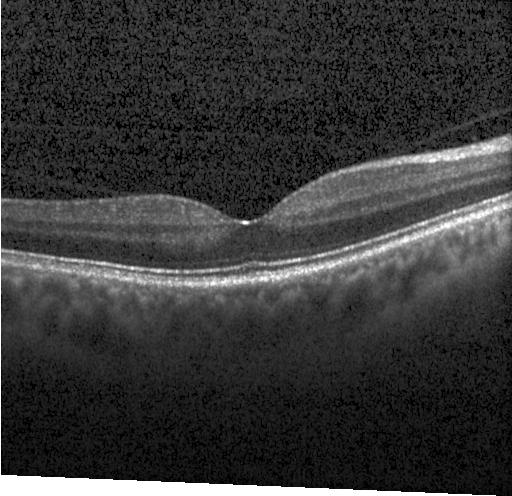
Finding: no choroidal neovascularization, no diabetic macular edema, and no drusen.